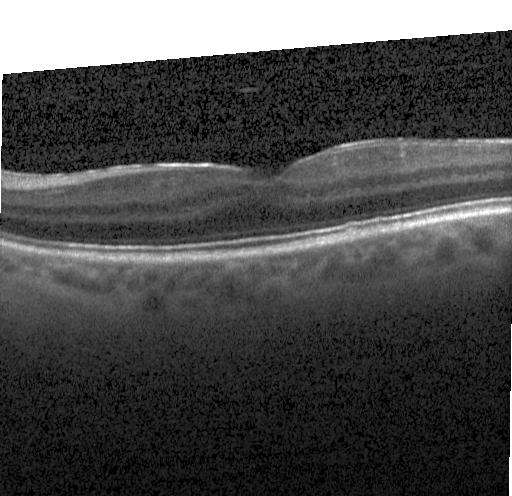

Heidelberg Spectralis OCT system · spectral-domain OCT · OCT B-scan
Assessment: no evidence of CNV, DME, or drusen.